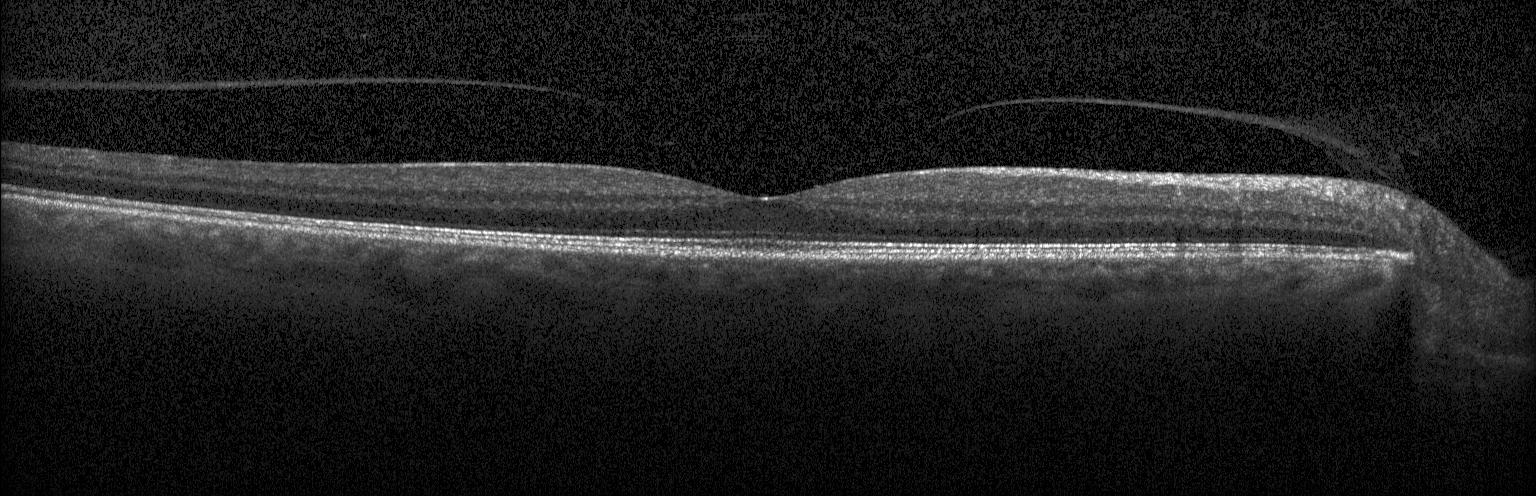
The scan shows neither choroidal neovascularization, diabetic macular edema, nor drusen.